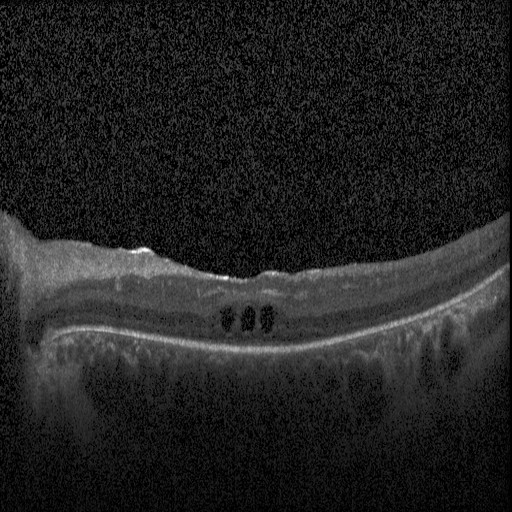 Optical coherence tomography B-scan — Macular OCT: diabetic macular edema.